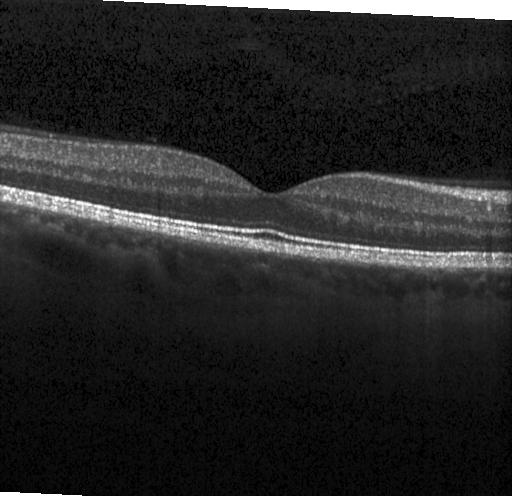
OCT B-scan, fovea-centered, Heidelberg Spectralis OCT system — Diagnosis: no CNV, DME, or drusen.